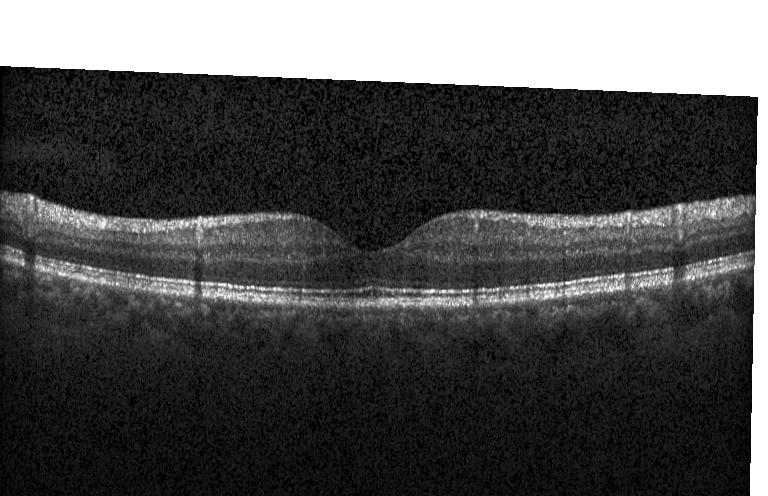

OCT B-scan
The scan shows neither CNV, DME, nor drusen.